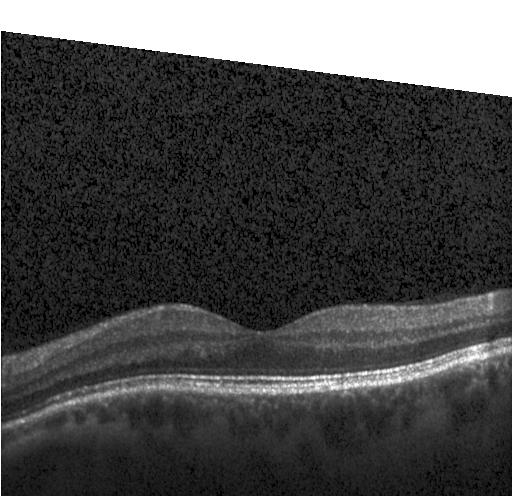
OCT line scan.
Diagnosis: no evidence of CNV, DME, or drusen.